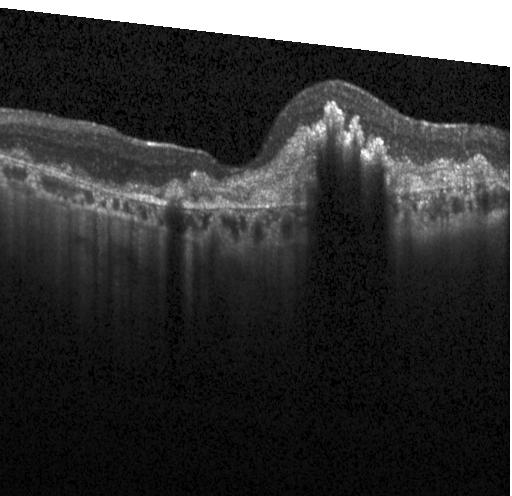 Macular OCT demonstrating a choroidal neovascular membrane.